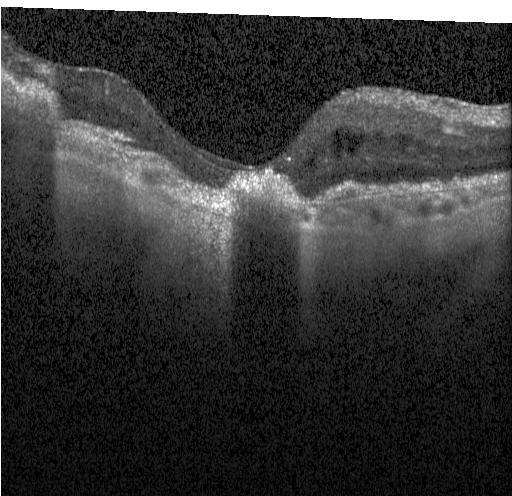 This B-scan demonstrates a choroidal neovascular membrane.